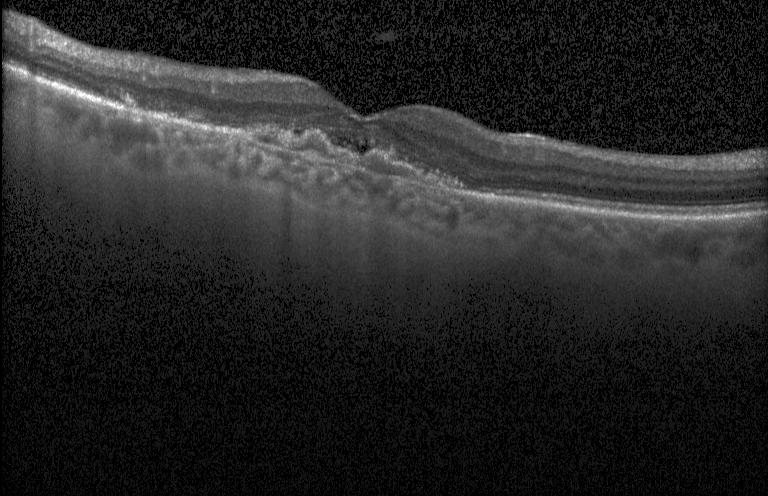

OCT line scan; through the macula; spectral-domain OCT
The scan shows choroidal neovascularization (CNV).